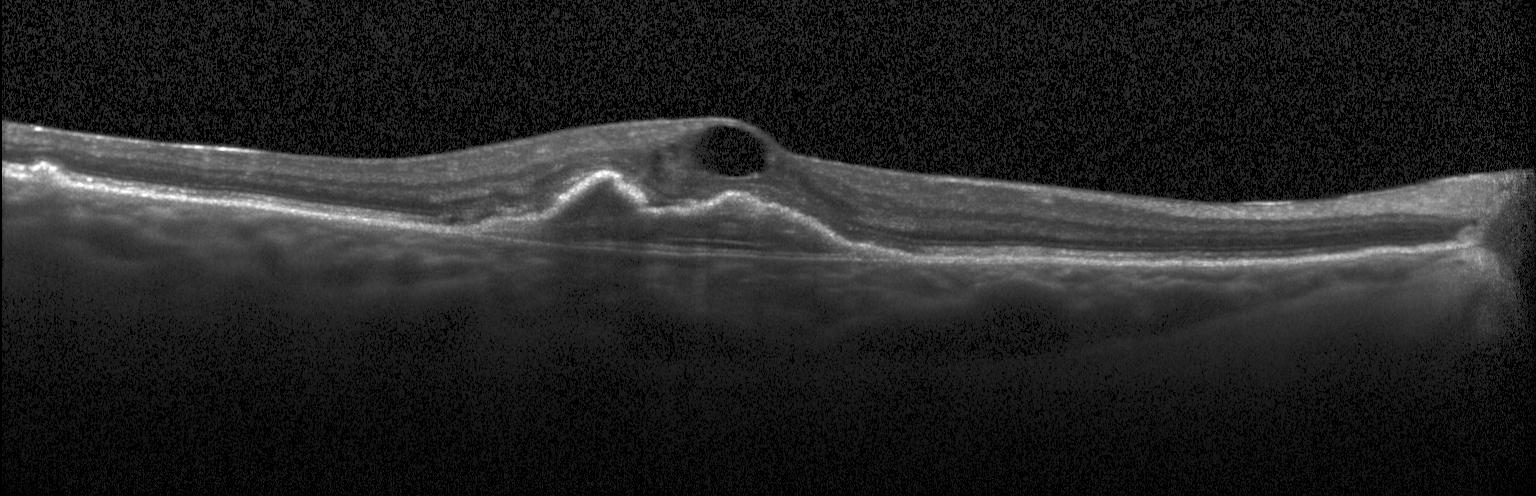 Retinal OCT cross-section, Heidelberg Spectralis OCT system. Finding: a choroidal neovascular membrane.